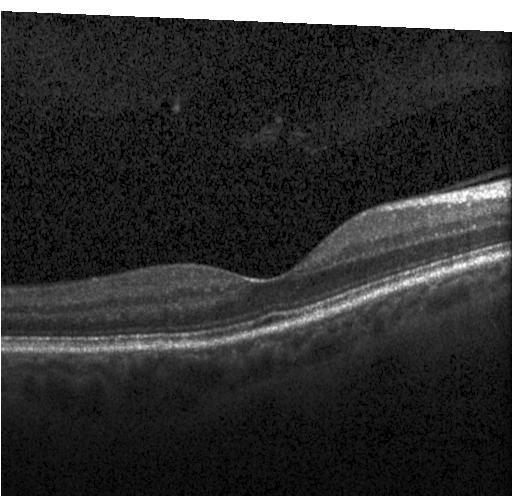 Retinal OCT cross-section showing neither choroidal neovascularization, diabetic macular edema, nor drusen.